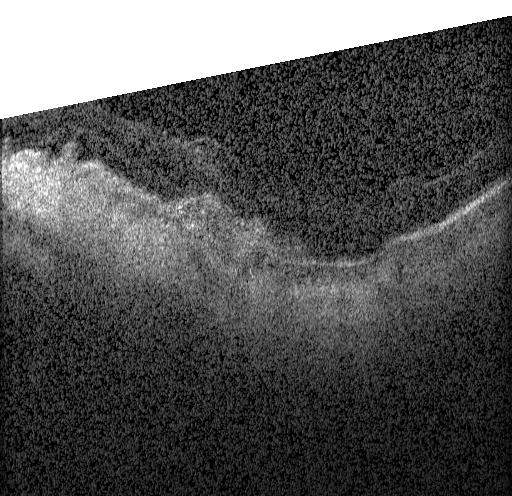

Assessment: a choroidal neovascular membrane.